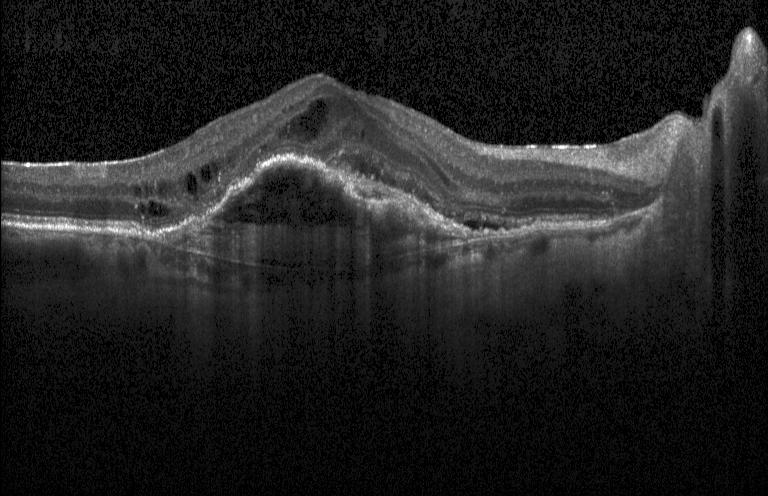

A choroidal neovascular membrane.